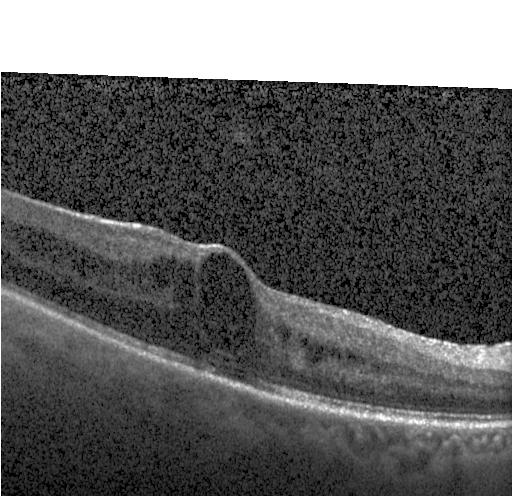 Centered on the fovea. Instrument: Heidelberg Spectralis. OCT line scan — Dx: diabetic macular edema.